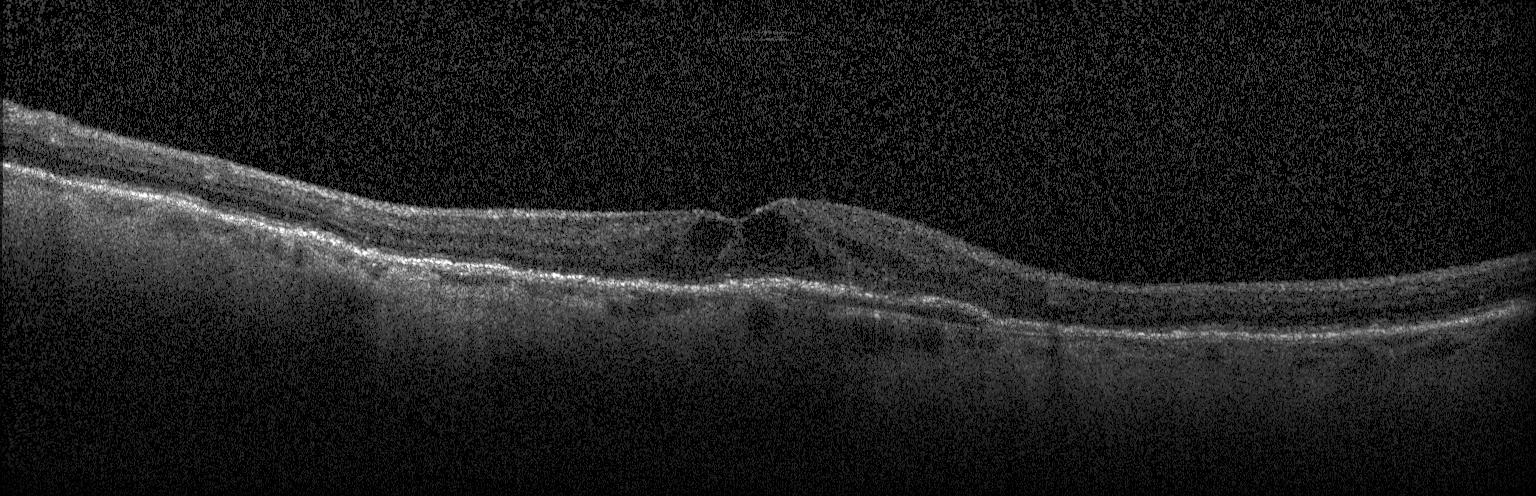
Macular scan · spectral-domain OCT · retinal OCT B-scan — Diagnosis: a choroidal neovascular membrane.